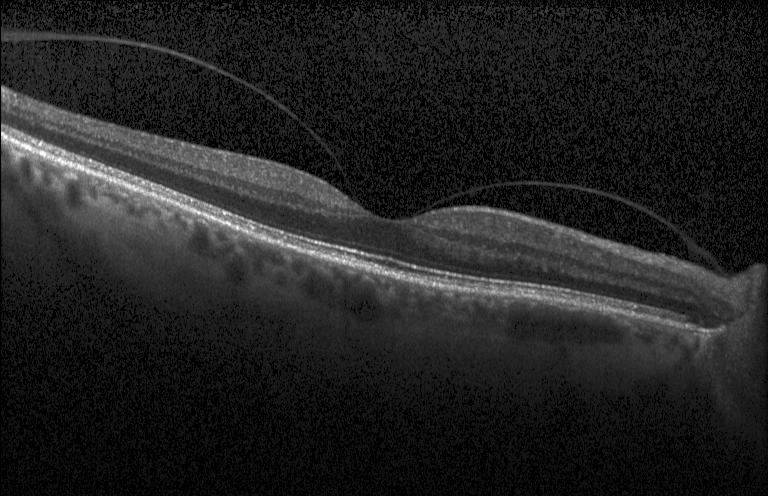
SD-OCT, optical coherence tomography B-scan.
No evidence of choroidal neovascularization, diabetic macular edema, or drusen.